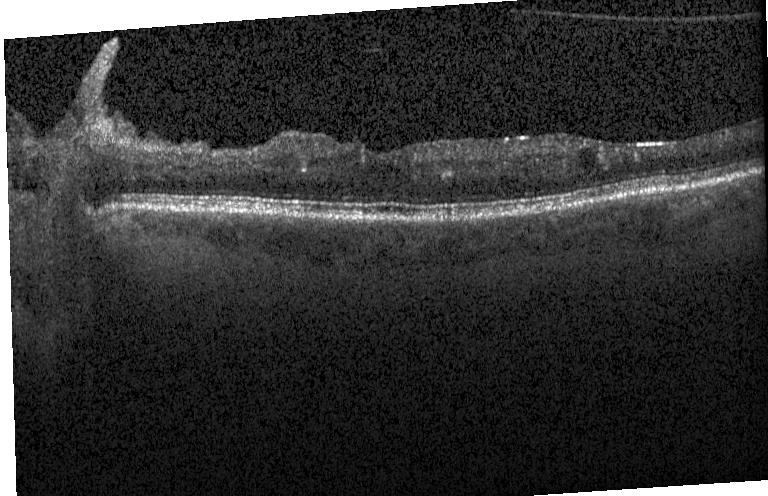

Heidelberg Spectralis, optical coherence tomography scan, SD-OCT
This B-scan demonstrates diabetic macular edema.